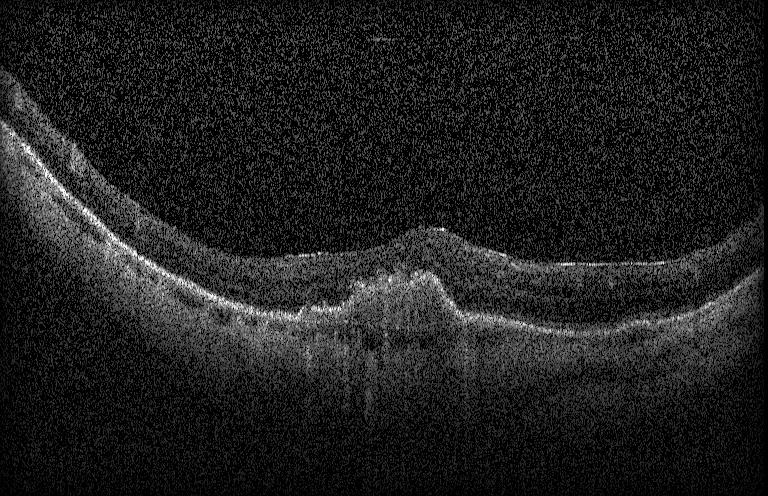

Spectral-domain optical coherence tomography · through the macula · Heidelberg Spectralis · OCT line scan.
Assessment: a choroidal neovascular membrane.